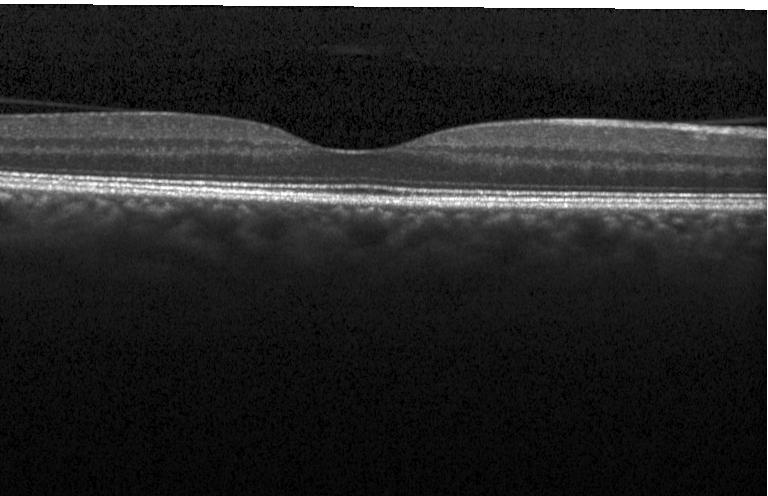

Macular OCT: no choroidal neovascularization, diabetic macular edema, or drusen.